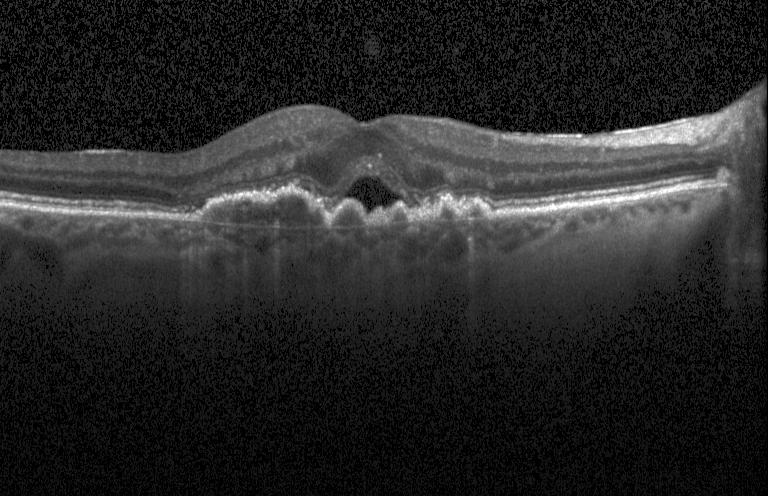 Spectral-domain optical coherence tomography · Heidelberg Spectralis · optical coherence tomography B-scan. Diagnosis: CNV.